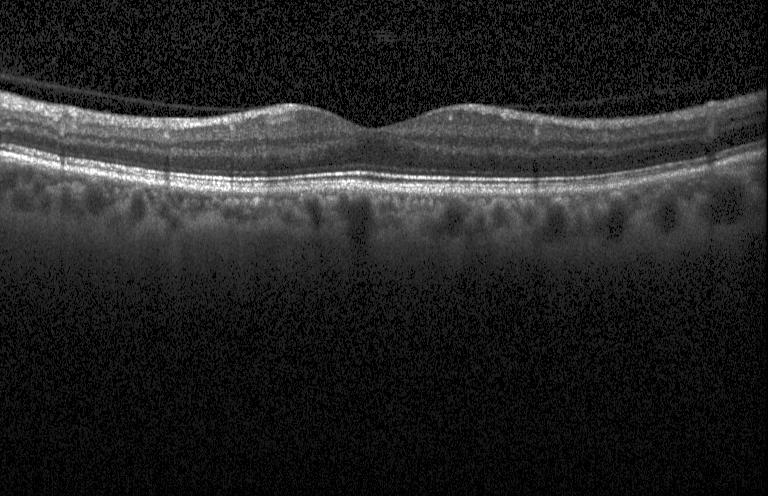
Finding: no CNV, DME, or drusen.